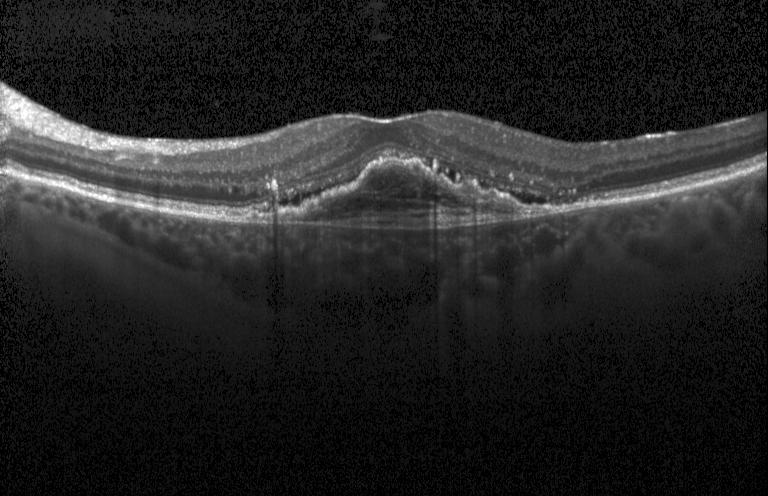 Assessment: choroidal neovascularization.